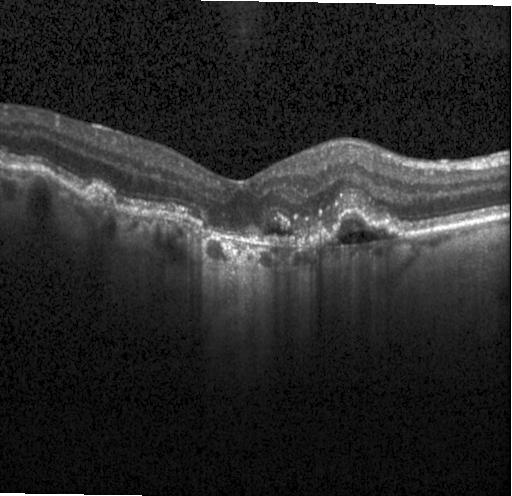

OCT B-scan; spectral-domain optical coherence tomography; Heidelberg Spectralis. OCT finding: a choroidal neovascular membrane.